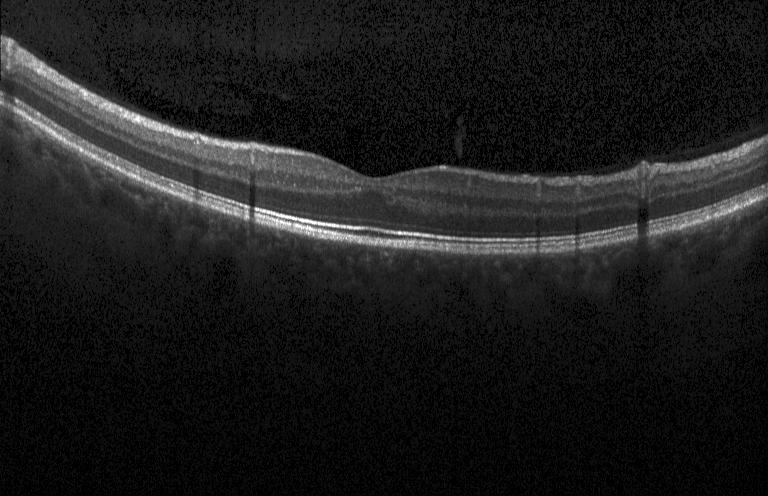
SD-OCT · Heidelberg Spectralis · optical coherence tomography scan · centered on the fovea
Dx: neither CNV, DME, nor drusen.